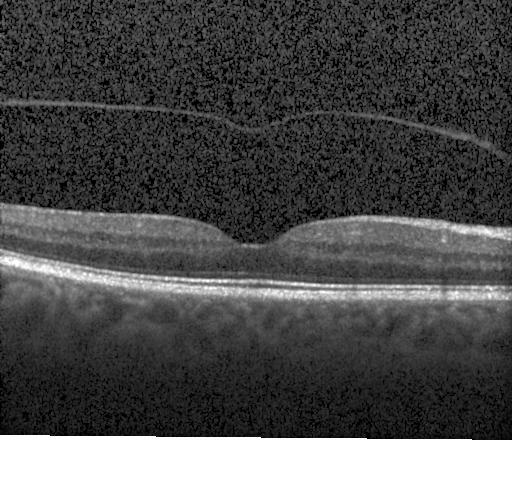

Fovea-centered. Retinal OCT cross-section
Dx: no evidence of choroidal neovascularization, diabetic macular edema, or drusen.